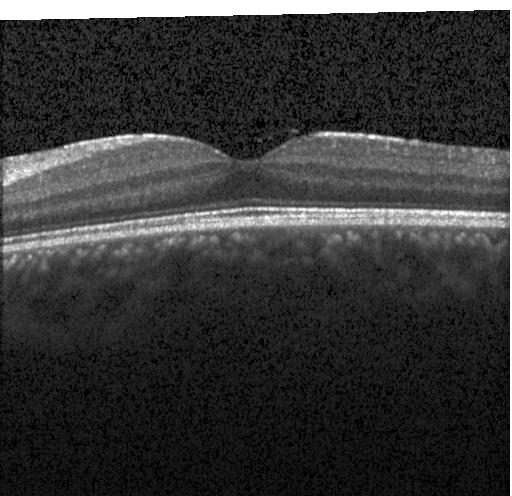
OCT B-scan showing no choroidal neovascularization, no diabetic macular edema, and no drusen.